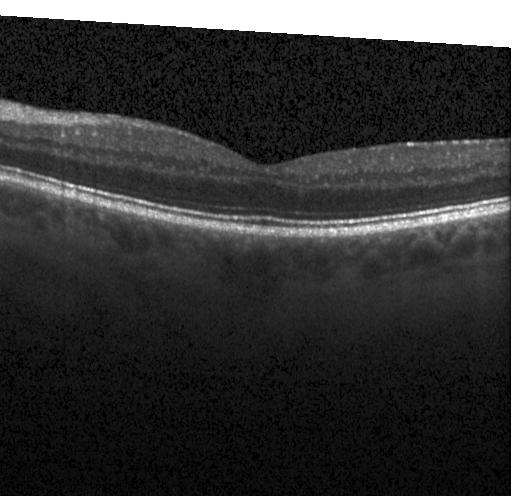 Retinal OCT cross-section; fovea-centered
This B-scan demonstrates neither CNV, DME, nor drusen.